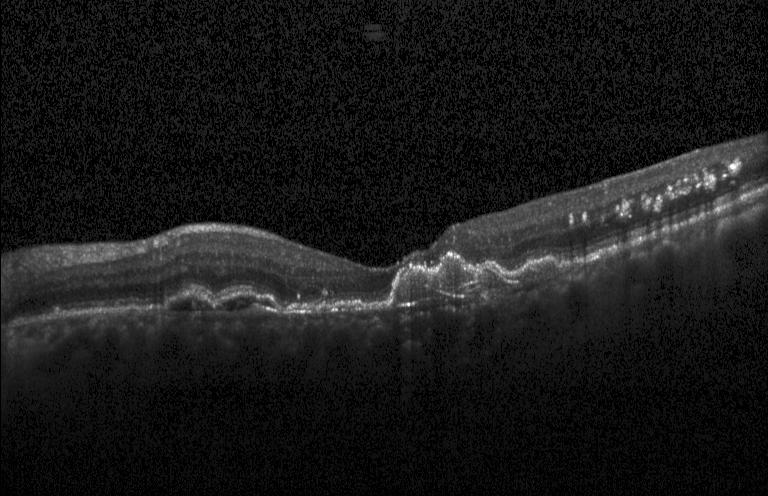

Finding: a choroidal neovascular membrane.